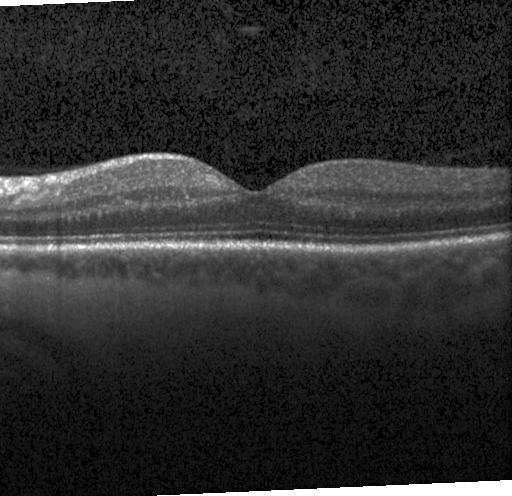

Assessment: no CNV, DME, or drusen.